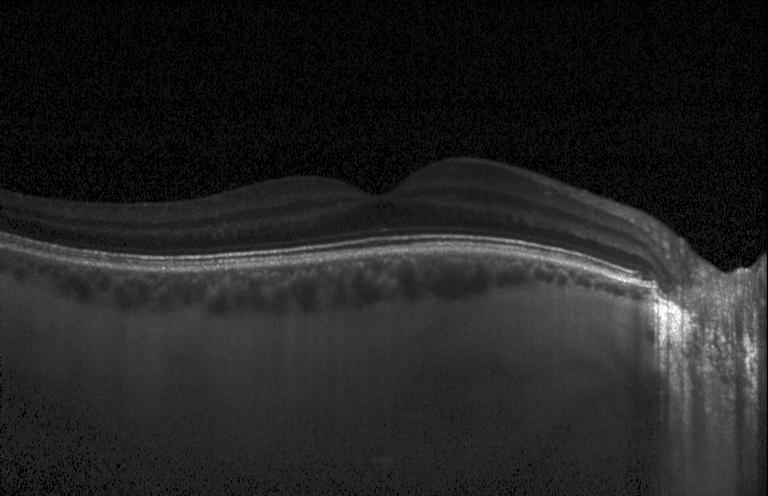
Assessment: no choroidal neovascularization, diabetic macular edema, or drusen.